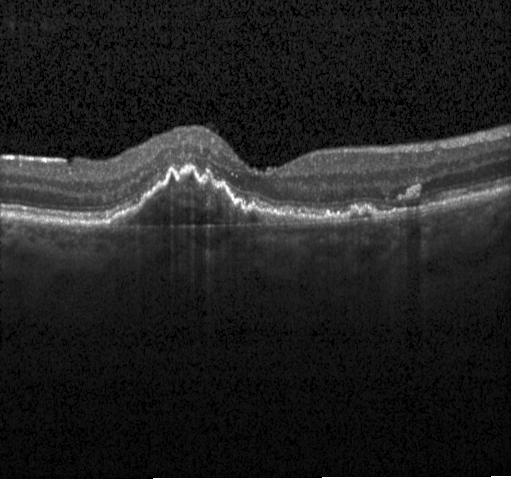

Optical coherence tomography scan, spectral-domain OCT, through the macula
Dx: a choroidal neovascular membrane.